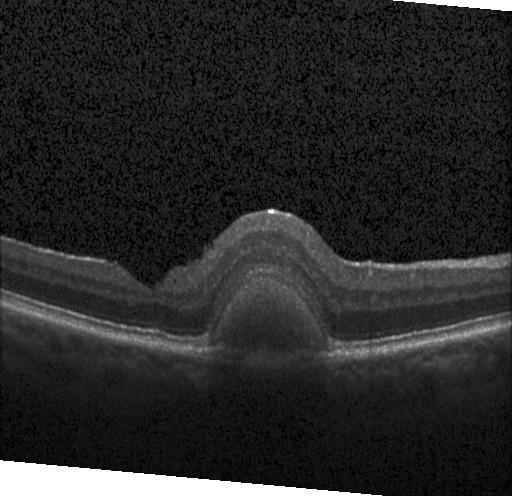 Optical coherence tomography B-scan · Heidelberg Spectralis · centered on the fovea — OCT finding: choroidal neovascularization (CNV).